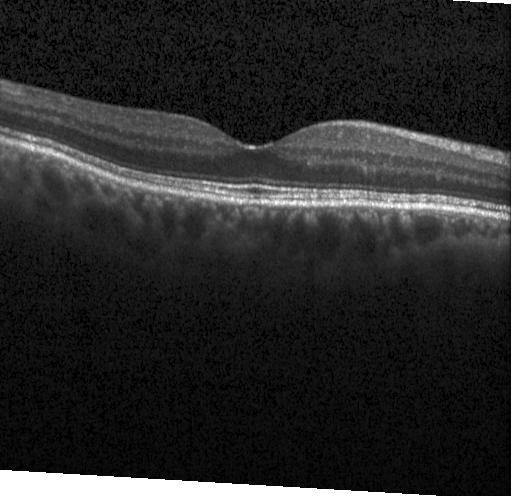 Retinal OCT B-scan. Assessment: no CNV, no DME, and no drusen.